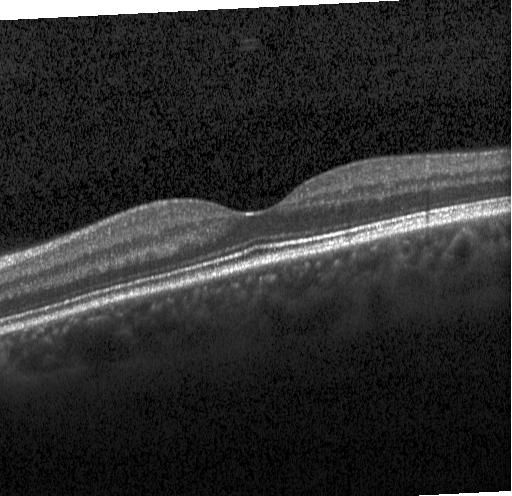

Spectral-domain optical coherence tomography · OCT line scan · Heidelberg Spectralis — This B-scan demonstrates no choroidal neovascularization, no diabetic macular edema, and no drusen.